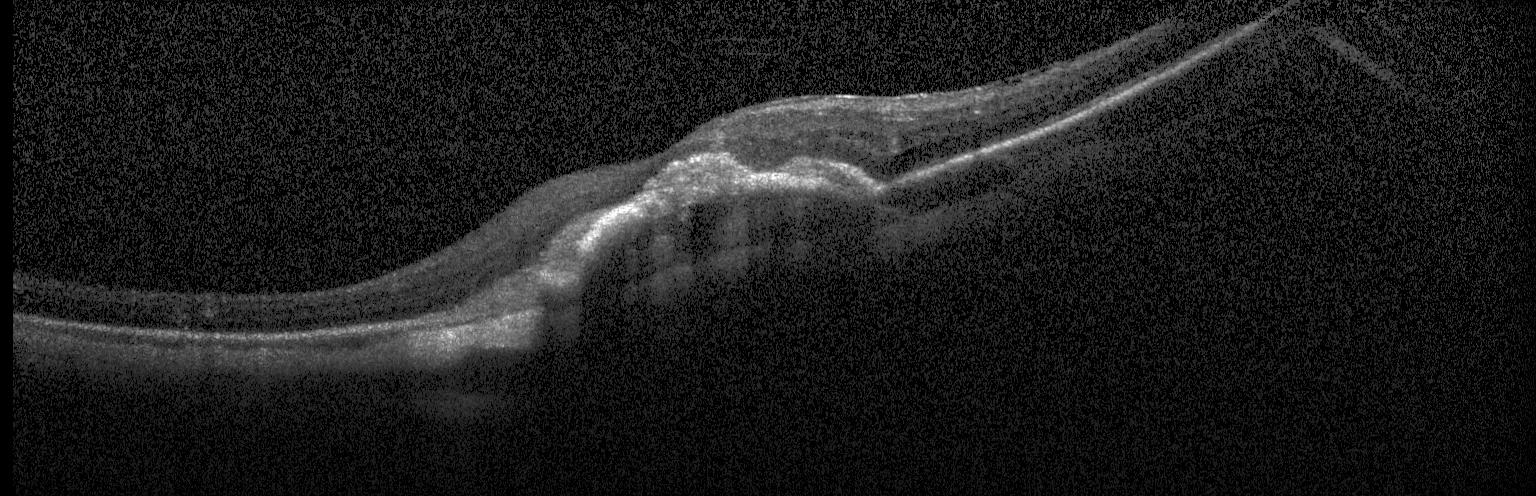
Finding: choroidal neovascularization (CNV).